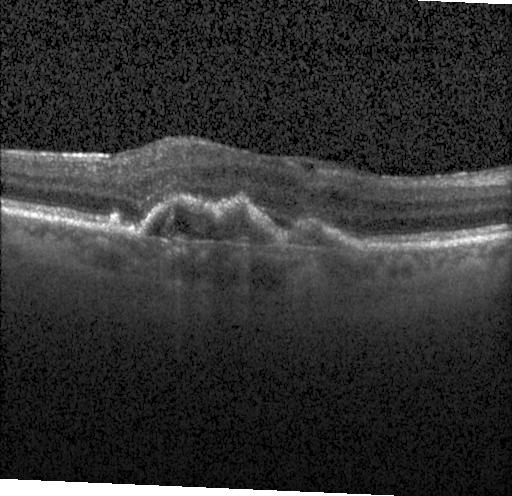 Macular OCT demonstrating a choroidal neovascular membrane.